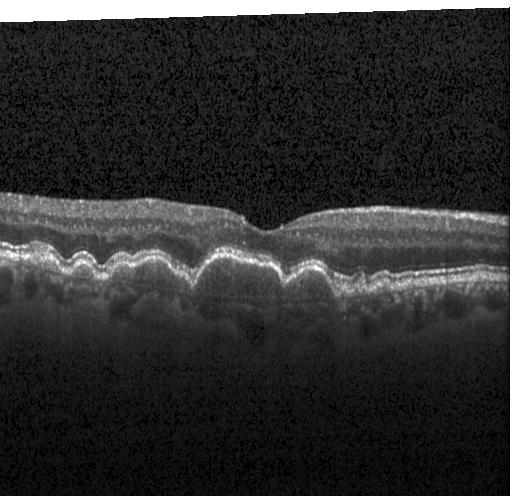

Diagnosis: multiple drusen.